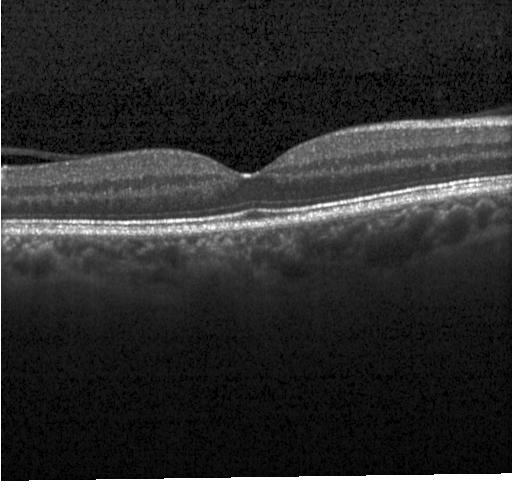 Optical coherence tomography scan. Impression: neither CNV, DME, nor drusen.